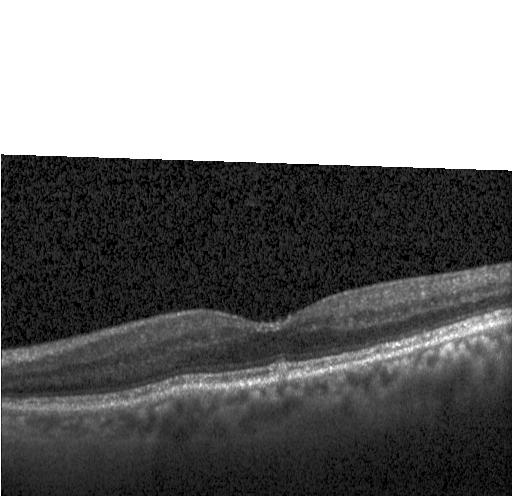

Spectral-domain OCT. Retinal OCT B-scan. Assessment: no CNV, DME, or drusen.